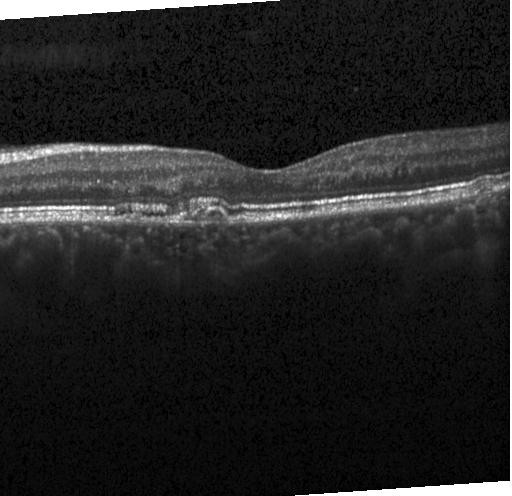
Macular OCT: a choroidal neovascular membrane.